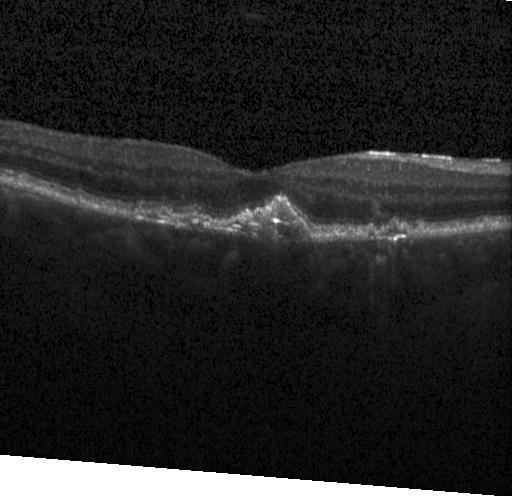

Centered on the fovea, retinal OCT B-scan, instrument: Heidelberg Spectralis. Impression: choroidal neovascularization.